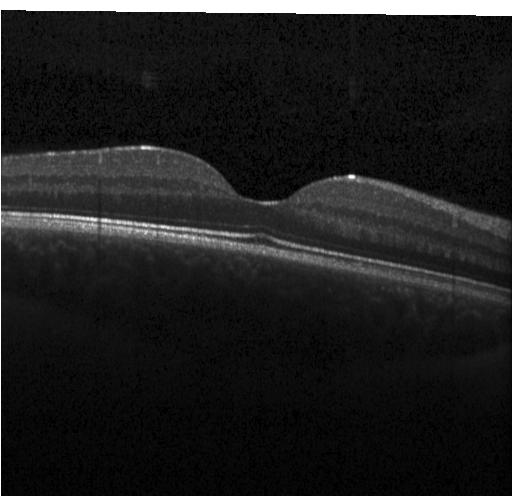 OCT finding: no choroidal neovascularization, diabetic macular edema, or drusen.